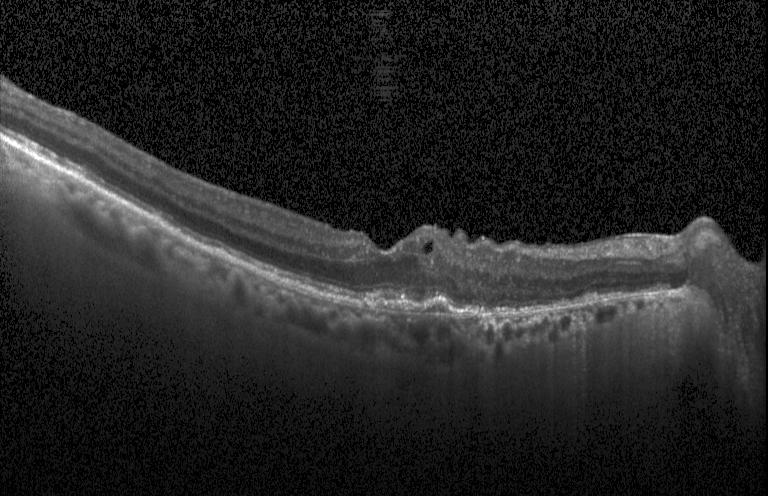

SD-OCT, Heidelberg Spectralis, fovea-centered, retinal OCT cross-section.
Diagnosis: choroidal neovascularization (CNV).